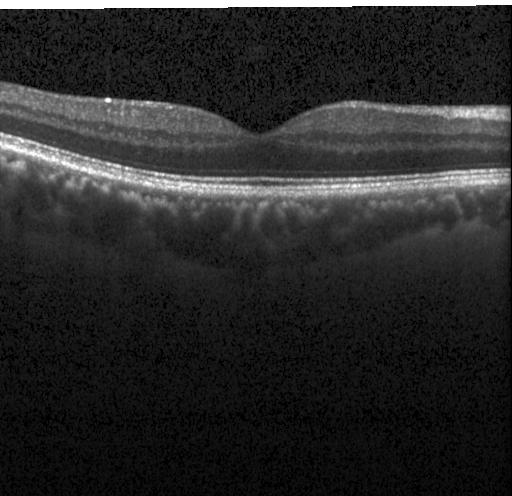

OCT B-scan — Diagnosis: no CNV, no DME, and no drusen.